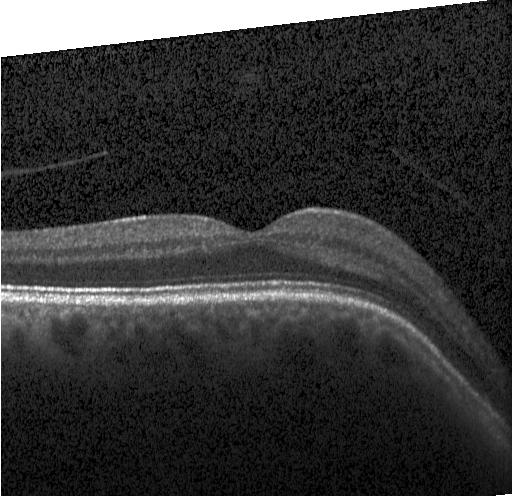 Centered on the fovea · OCT B-scan.
Finding: no choroidal neovascularization, diabetic macular edema, or drusen.